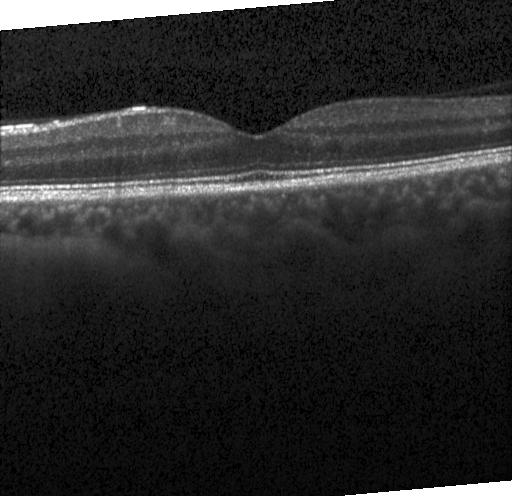

This B-scan demonstrates no evidence of choroidal neovascularization, diabetic macular edema, or drusen.